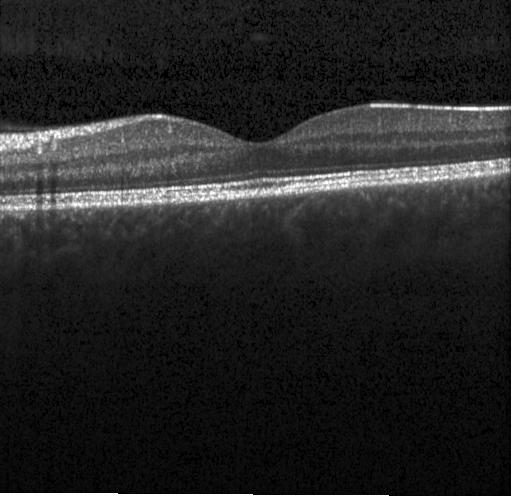
This B-scan demonstrates no evidence of choroidal neovascularization, diabetic macular edema, or drusen.